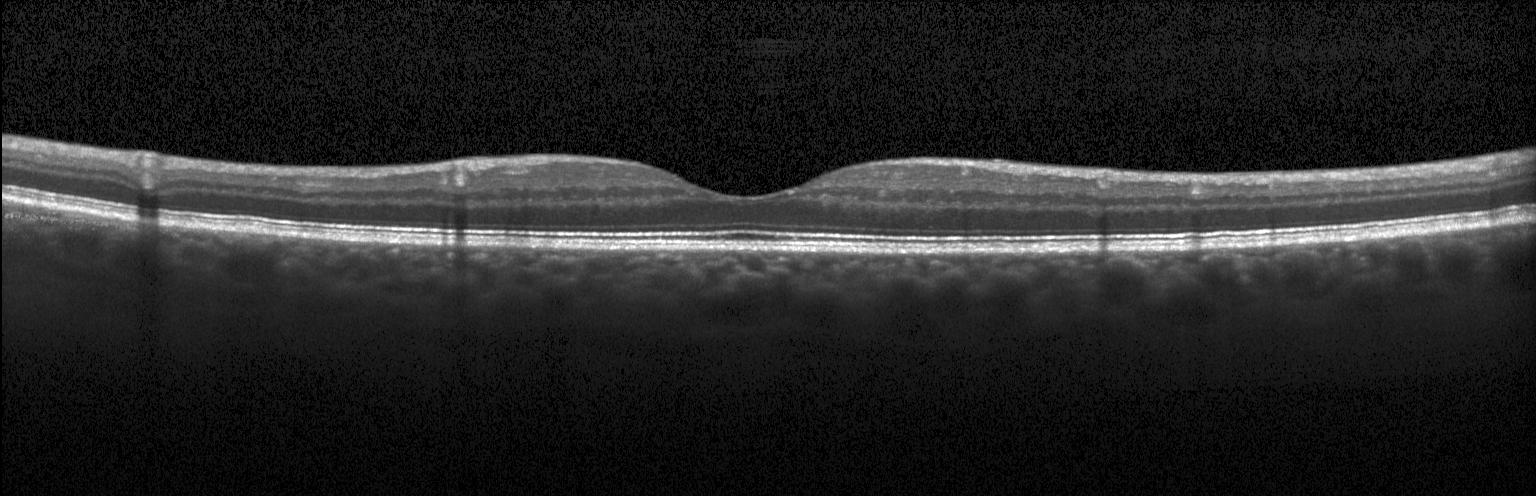

Fovea-centered. SD-OCT. Retinal OCT cross-section — This B-scan demonstrates no CNV, DME, or drusen.